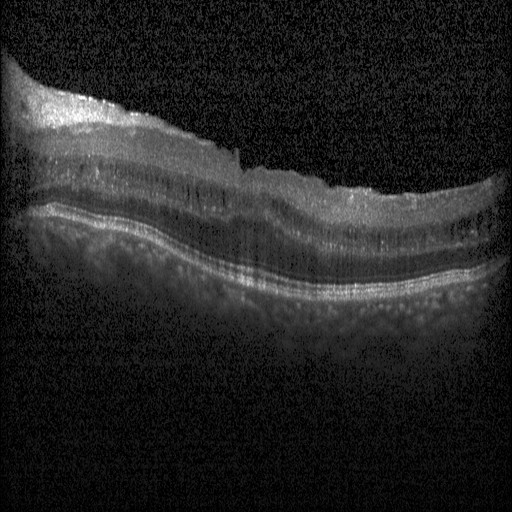
Optical coherence tomography scan · spectral-domain optical coherence tomography · horizontal scan through the fovea.
Diabetic macular edema.